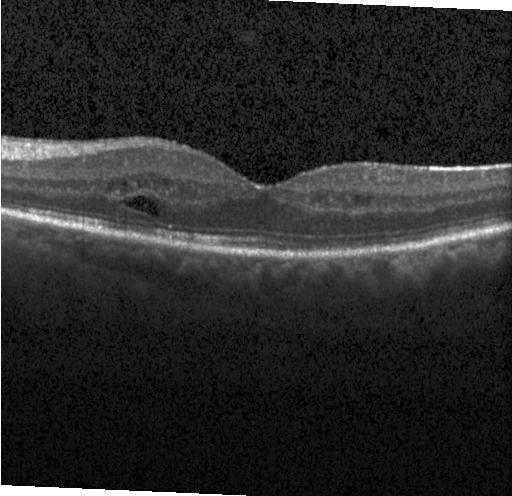
Assessment: DME.